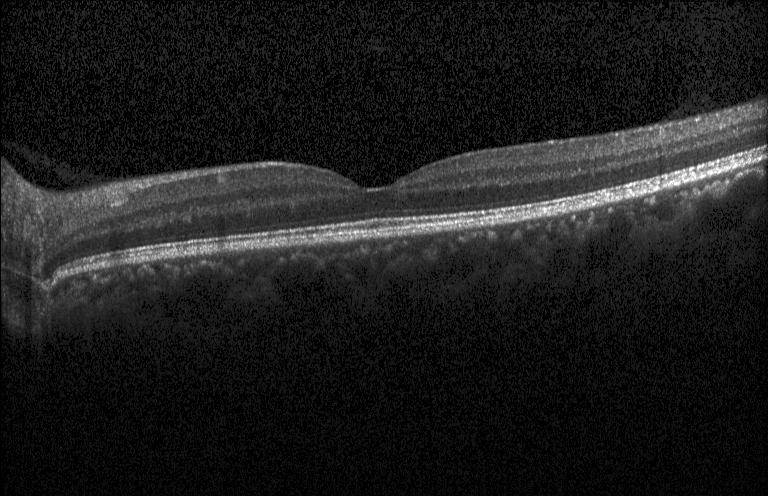

The scan shows no choroidal neovascularization, diabetic macular edema, or drusen.